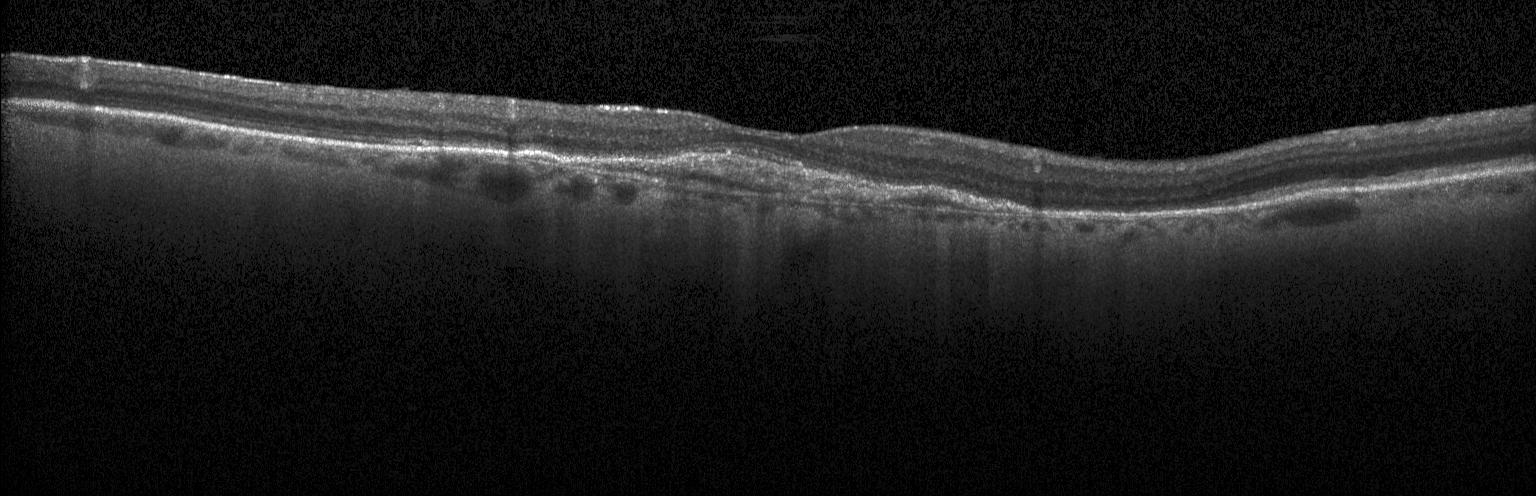

OCT B-scan · macular scan · Heidelberg Spectralis OCT system.
Assessment: choroidal neovascularization.